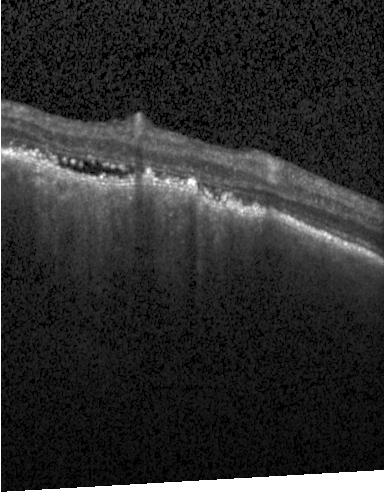

Finding: choroidal neovascularization.